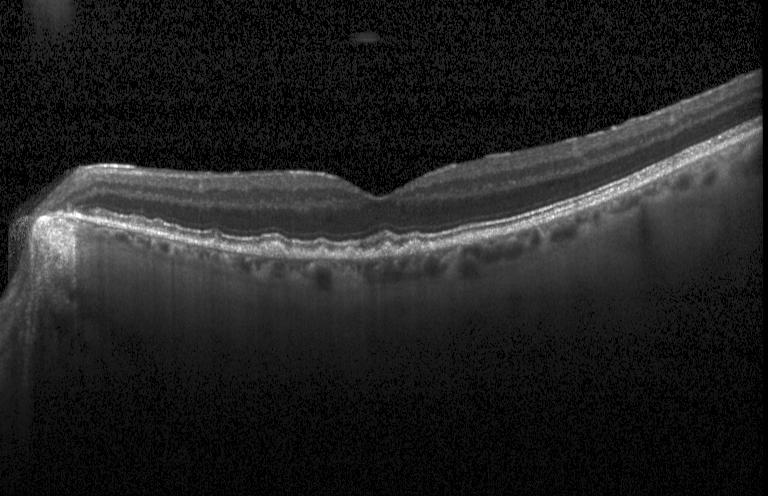

SD-OCT · OCT B-scan.
Multiple drusen.